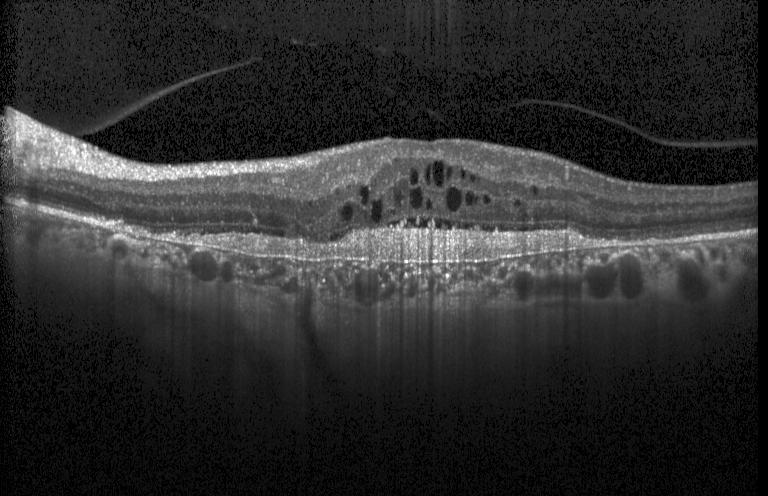
Finding: a choroidal neovascular membrane.